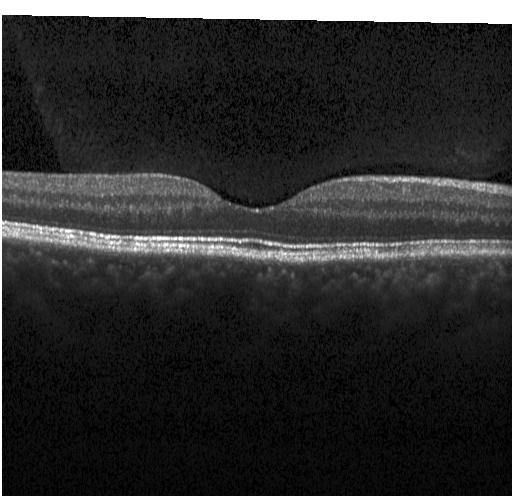

Optical coherence tomography B-scan
OCT finding: no choroidal neovascularization, diabetic macular edema, or drusen.